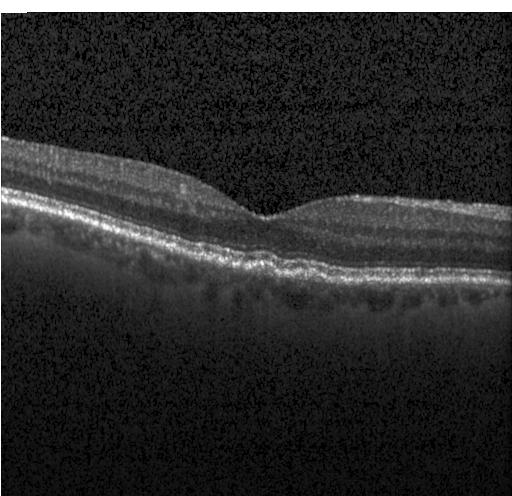 Retinal OCT cross-section showing drusen.